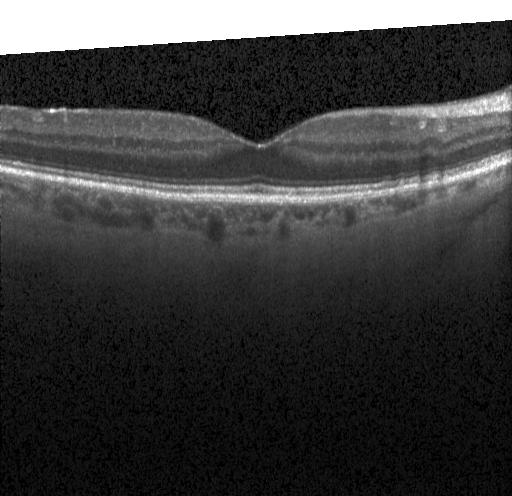
Retinal OCT B-scan. Centered on the fovea
Diagnosis: no choroidal neovascularization, diabetic macular edema, or drusen.